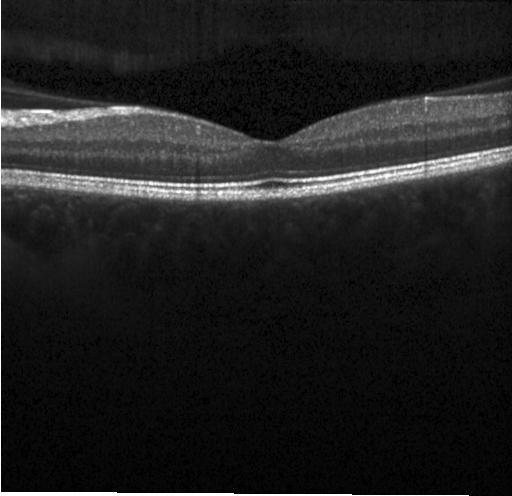

Neither choroidal neovascularization, diabetic macular edema, nor drusen.